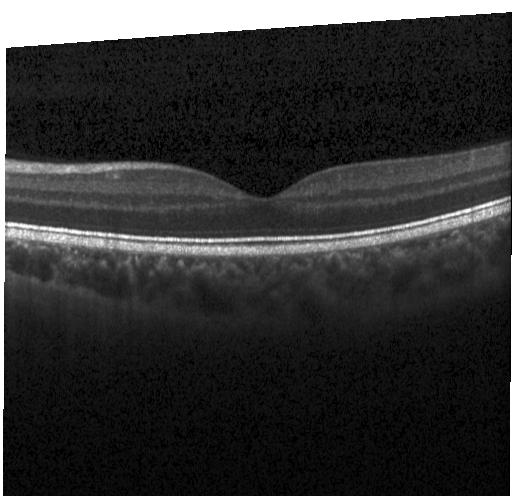
Finding: no evidence of choroidal neovascularization, diabetic macular edema, or drusen.